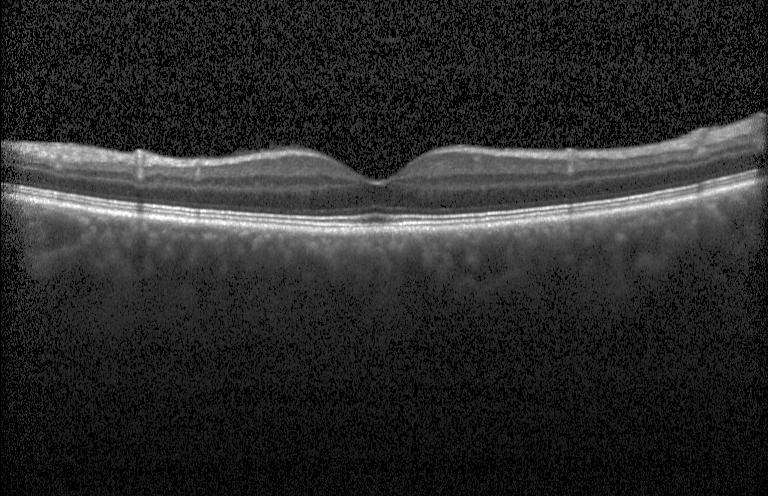
Through the macula · Heidelberg Spectralis · OCT B-scan · spectral-domain OCT — Macular OCT: neither choroidal neovascularization, diabetic macular edema, nor drusen.